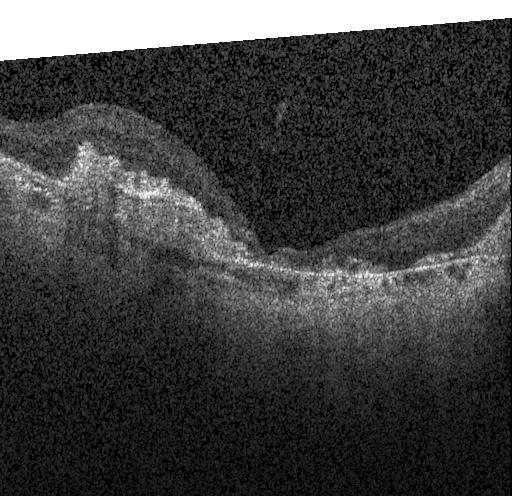 Finding: CNV.